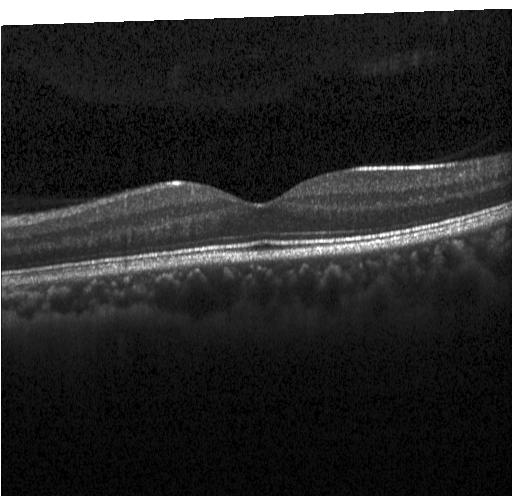 Optical coherence tomography scan. Acquired on a Heidelberg Spectralis. Spectral-domain optical coherence tomography. Macular scan
Diagnosis: no evidence of CNV, DME, or drusen.